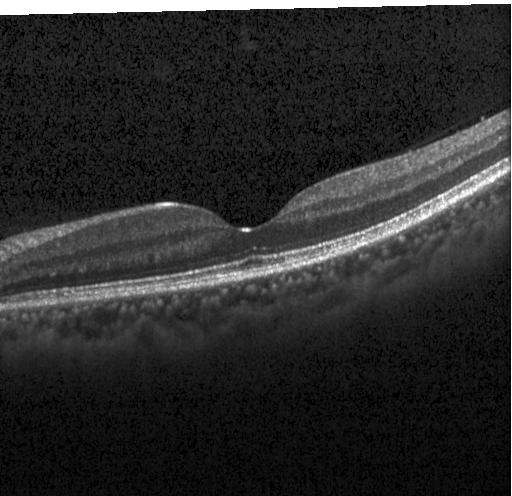

Acquired on a Heidelberg Spectralis · spectral-domain optical coherence tomography · optical coherence tomography scan
Macular OCT: no choroidal neovascularization, no diabetic macular edema, and no drusen.